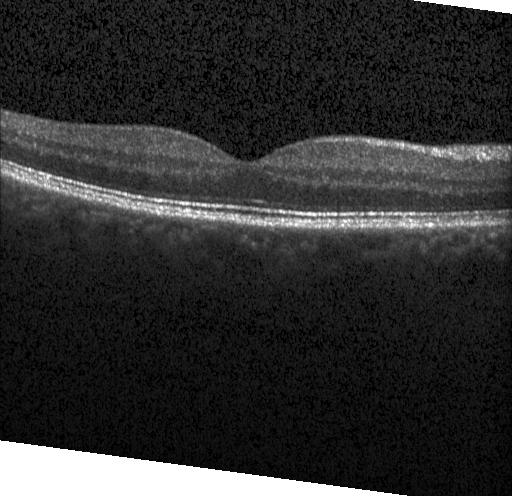
OCT finding: no evidence of CNV, DME, or drusen.